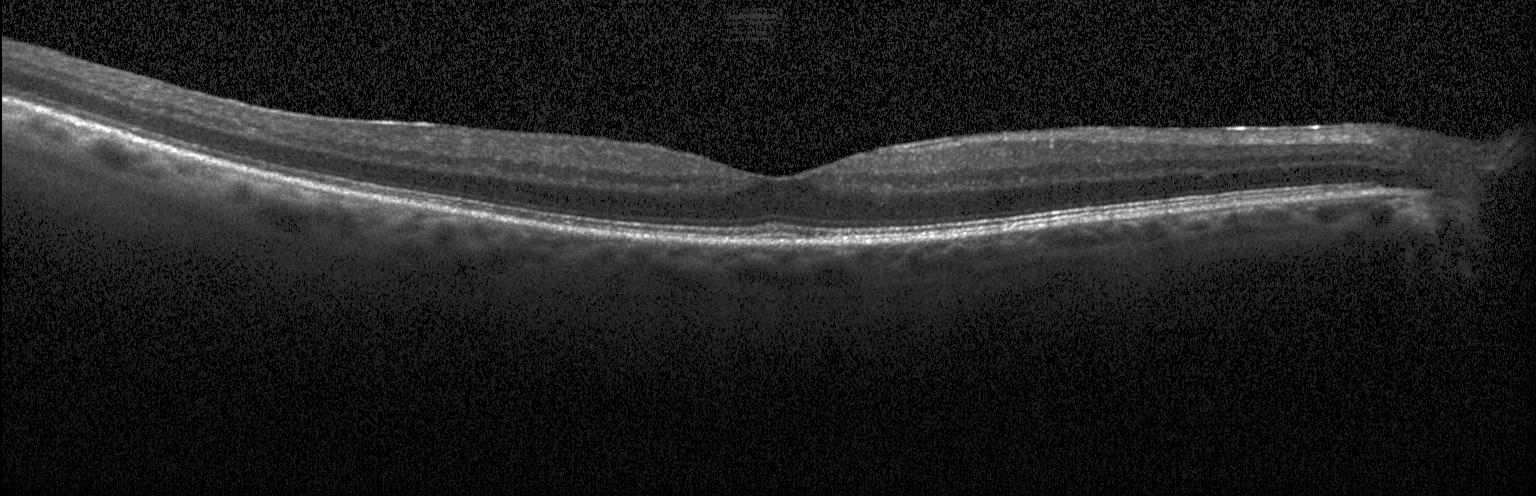 Optical coherence tomography scan. Acquired on a Heidelberg Spectralis. SD-OCT — No evidence of CNV, DME, or drusen.